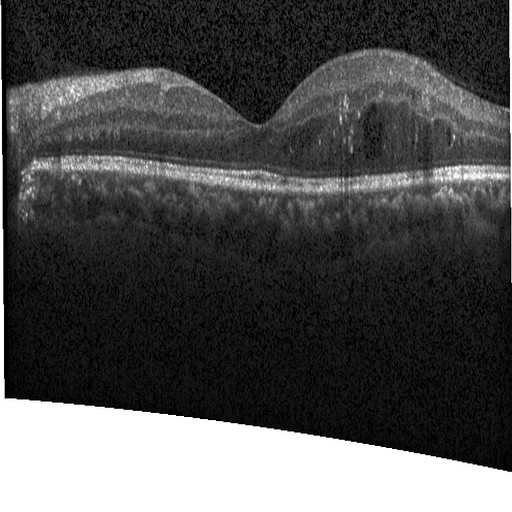 Finding: diabetic macular edema.